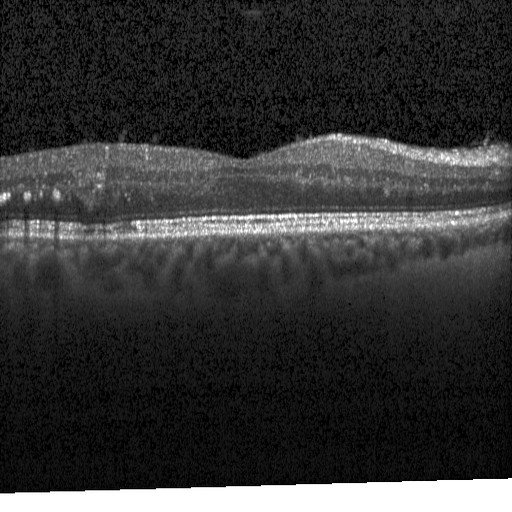

Macular OCT demonstrating diabetic macular edema (DME).